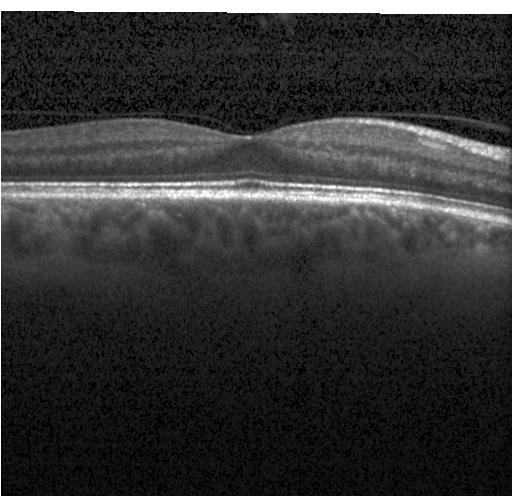

OCT B-scan; spectral-domain OCT; through the macula; acquired on a Heidelberg Spectralis.
Finding: no choroidal neovascularization, diabetic macular edema, or drusen.